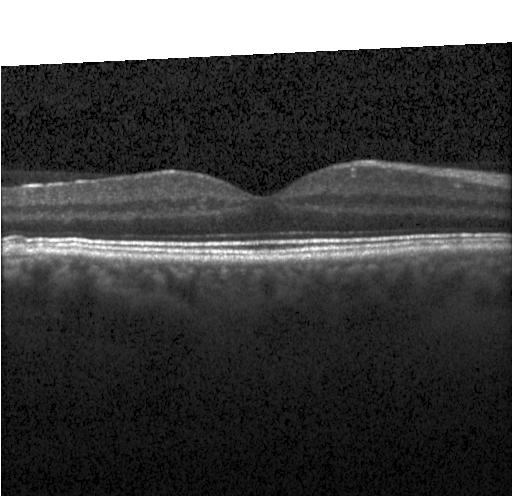 OCT B-scan.
Drusen.